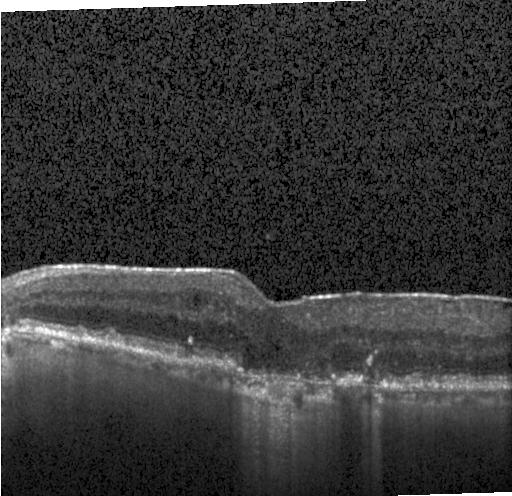 OCT line scan
Macular OCT: choroidal neovascularization (CNV).